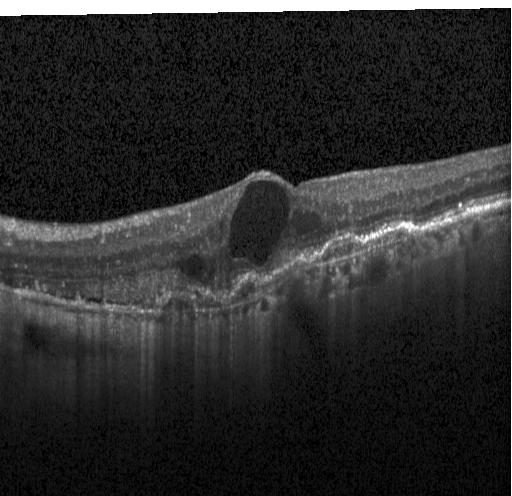 Instrument: Heidelberg Spectralis · fovea-centered · OCT line scan. Impression: a choroidal neovascular membrane.